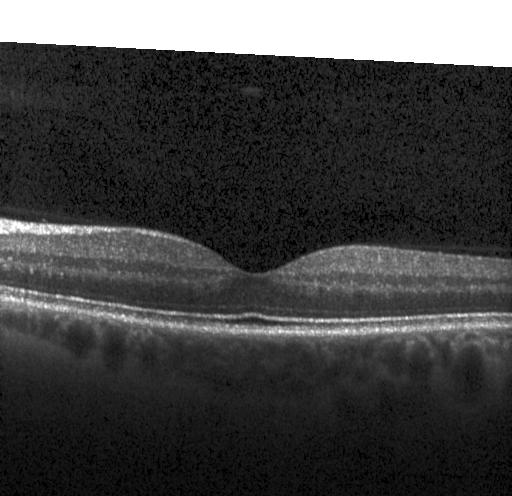
Impression: no CNV, DME, or drusen.